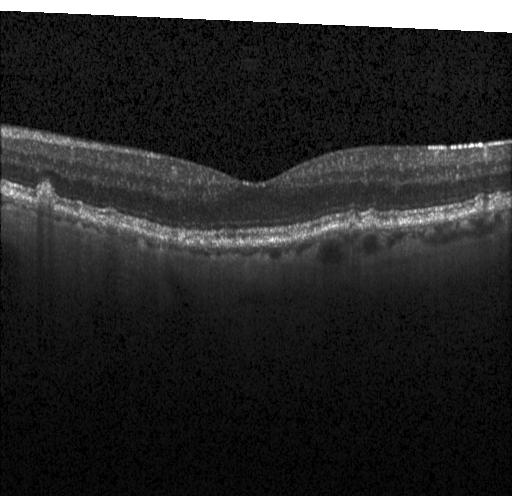 Finding: multiple drusen.